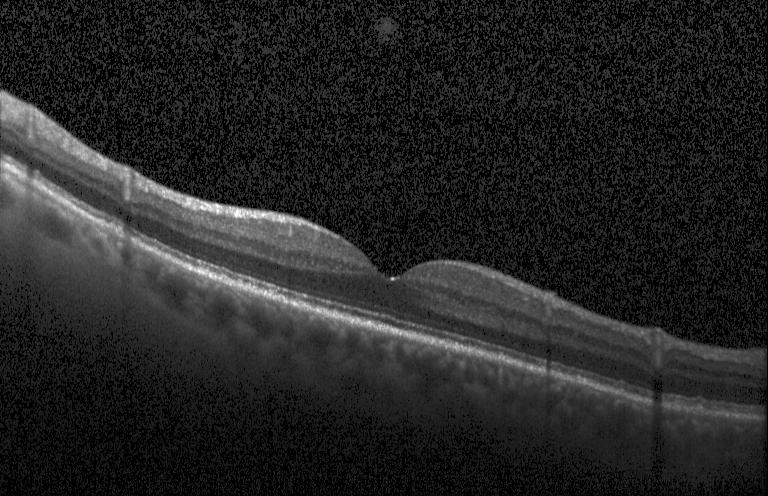 Retinal OCT B-scan.
Impression: drusen.